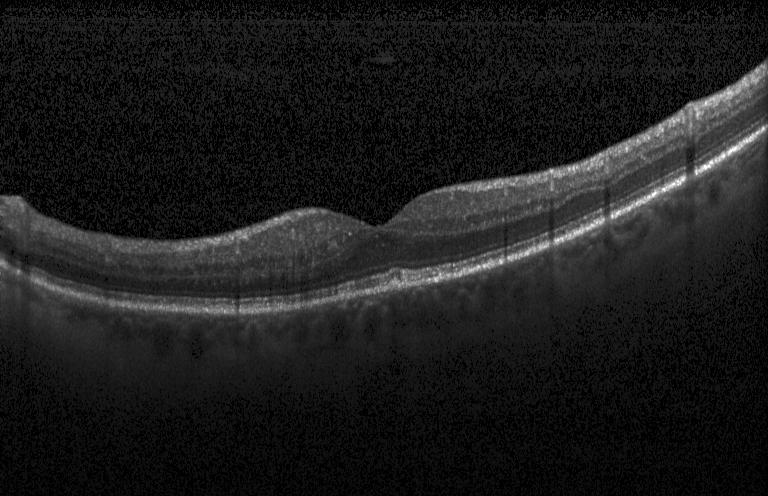

OCT B-scan
Dx: neither choroidal neovascularization, diabetic macular edema, nor drusen.